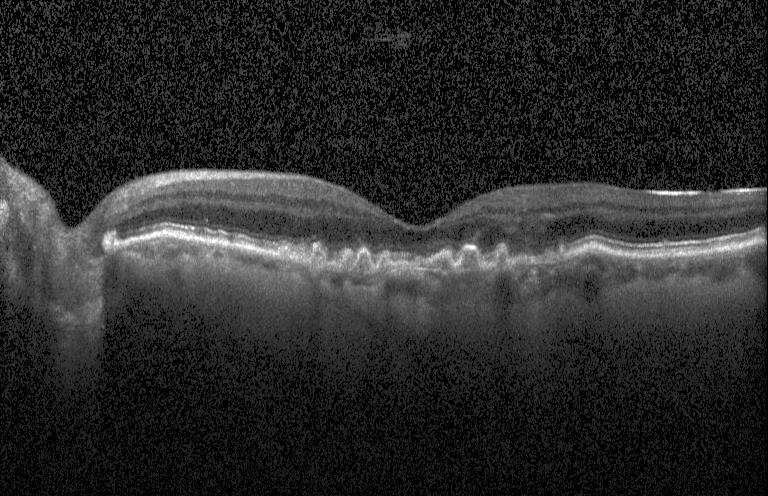 Retinal OCT B-scan
Macular OCT: multiple drusen.